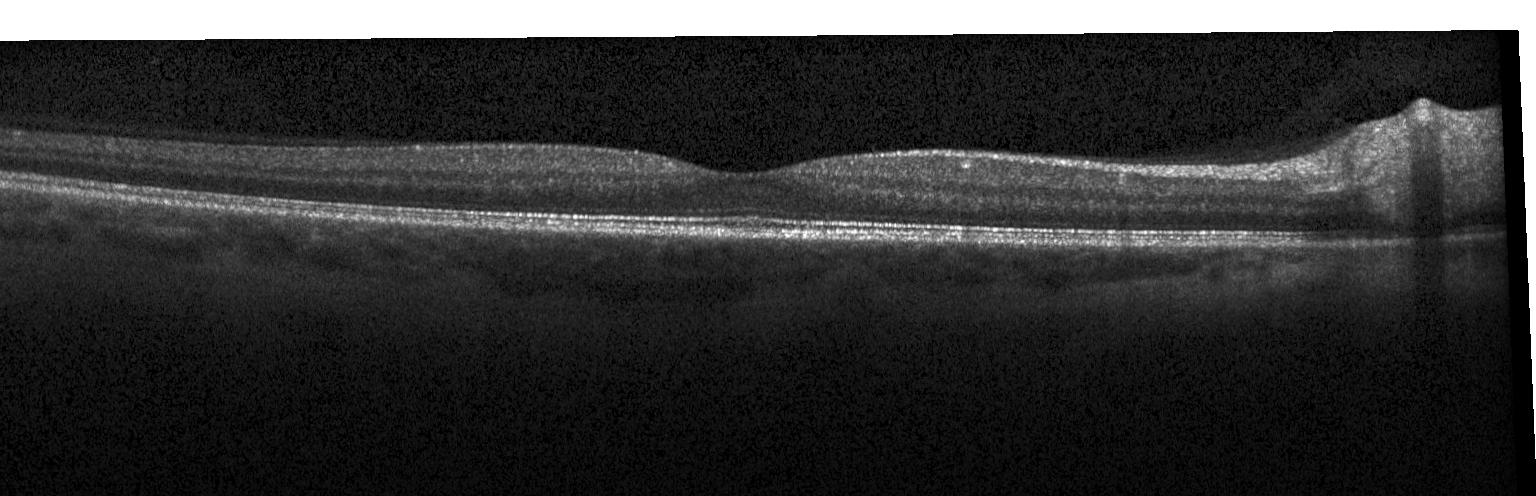

Retinal OCT cross-section showing no evidence of choroidal neovascularization, diabetic macular edema, or drusen.